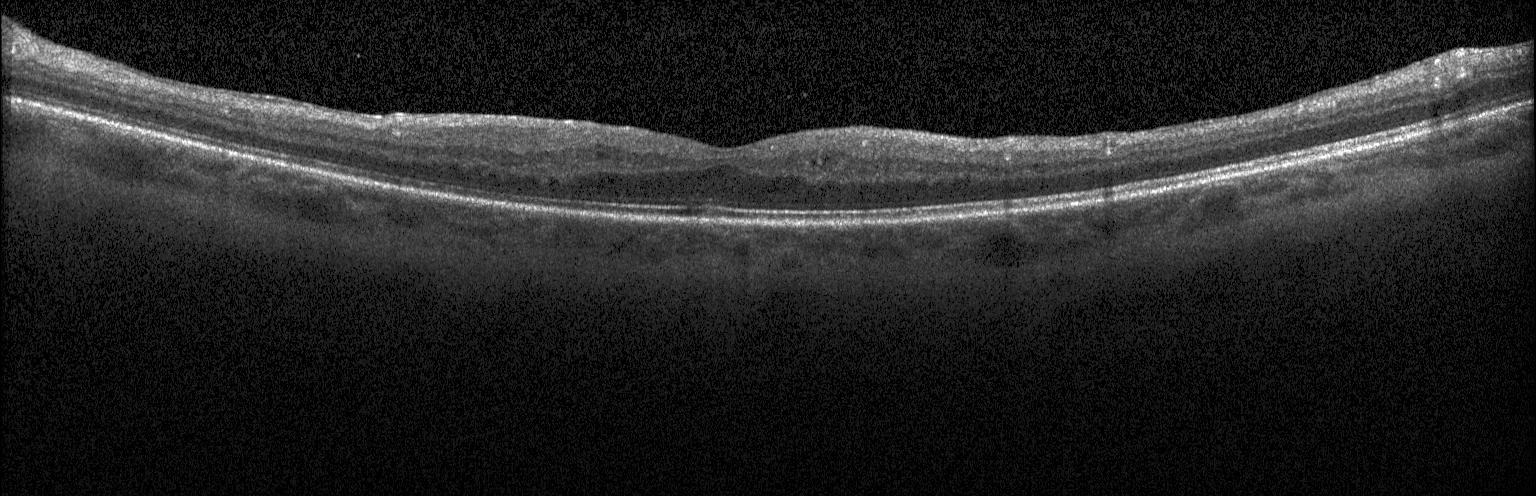 Optical coherence tomography B-scan, SD-OCT — Impression: diabetic macular edema (DME).